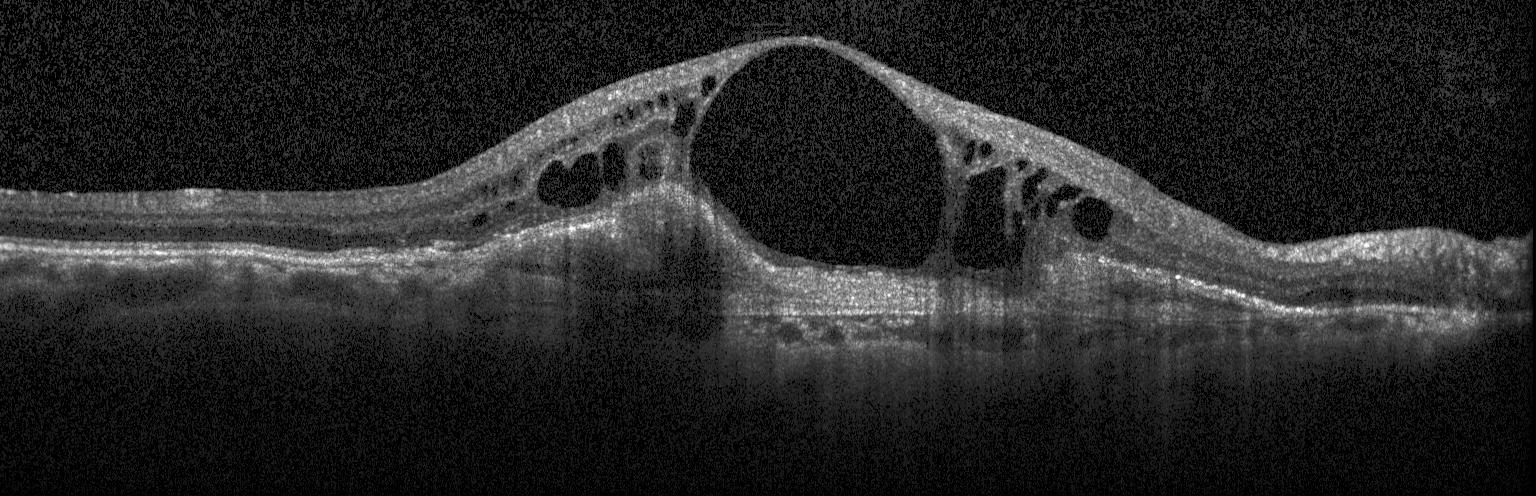 The scan shows a choroidal neovascular membrane.